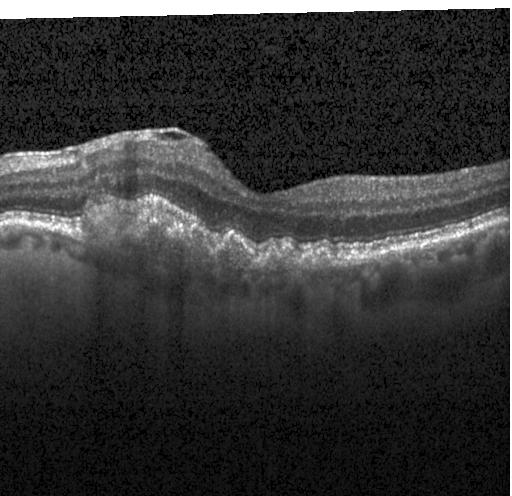
The scan shows CNV.